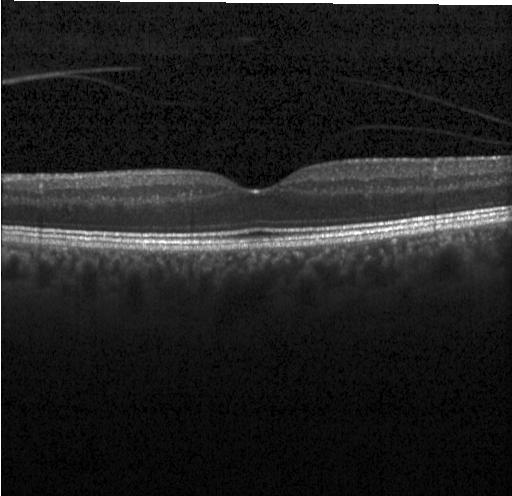

Macular OCT: no choroidal neovascularization, no diabetic macular edema, and no drusen.